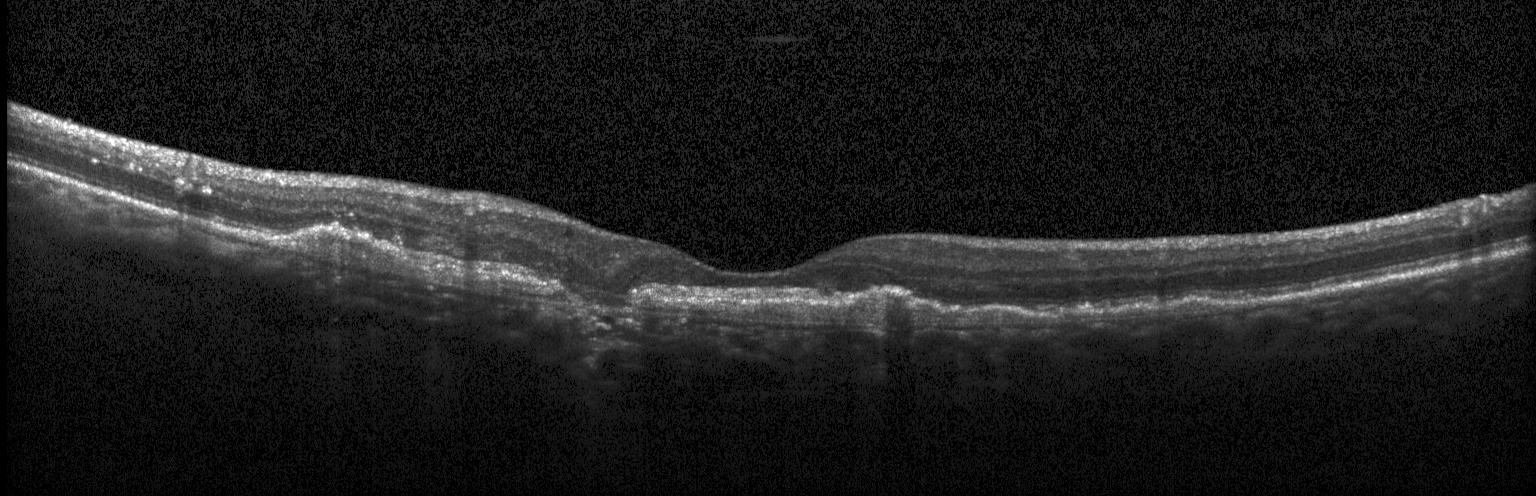 Macular OCT: a choroidal neovascular membrane.